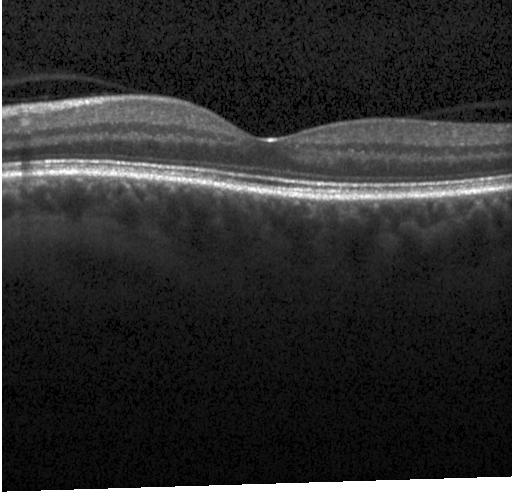 SD-OCT. Optical coherence tomography B-scan. Horizontal scan through the fovea. Acquired on a Heidelberg Spectralis.
This B-scan demonstrates no evidence of CNV, DME, or drusen.